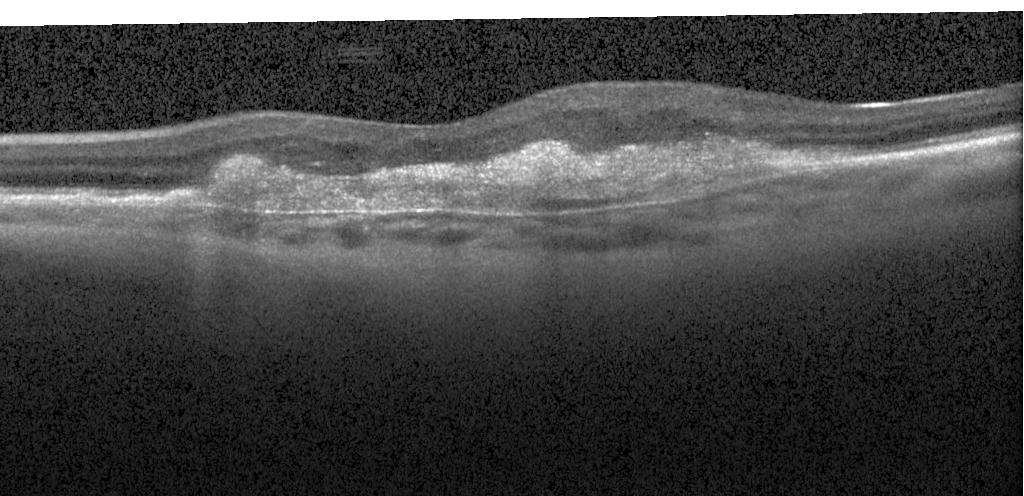

Optical coherence tomography scan, fovea-centered — OCT finding: choroidal neovascularization (CNV).